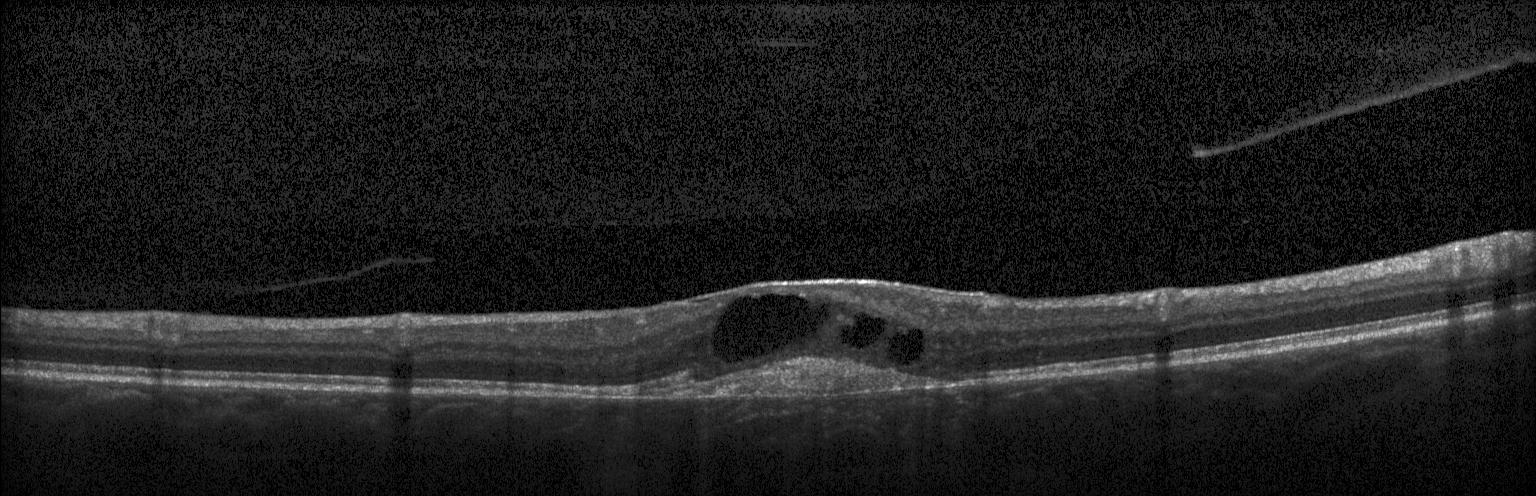 SD-OCT, optical coherence tomography B-scan, centered on the fovea, instrument: Heidelberg Spectralis
Impression: choroidal neovascularization.